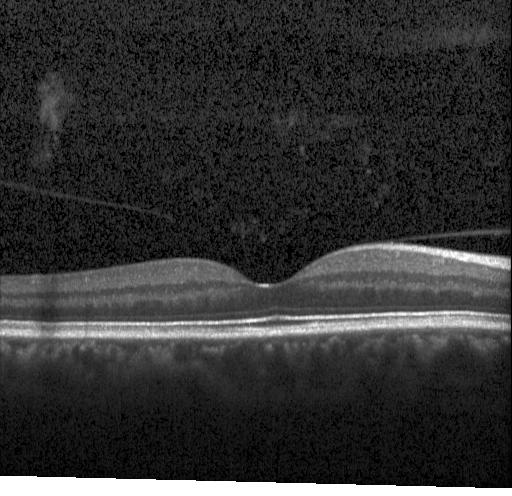 OCT B-scan showing neither choroidal neovascularization, diabetic macular edema, nor drusen.